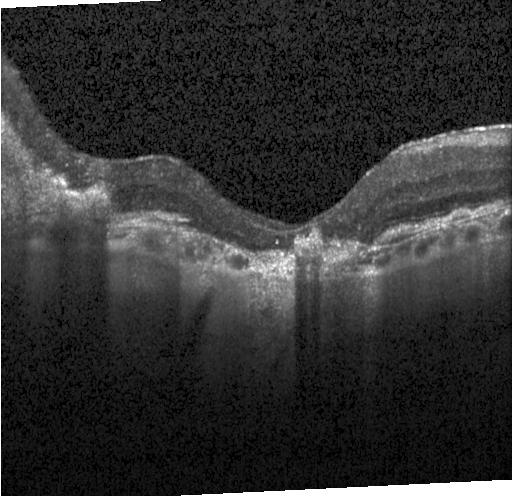 Optical coherence tomography scan.
A choroidal neovascular membrane.